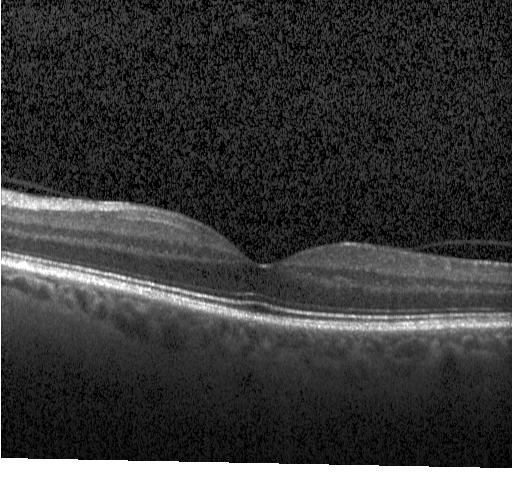

SD-OCT; optical coherence tomography scan.
Diagnosis: neither choroidal neovascularization, diabetic macular edema, nor drusen.